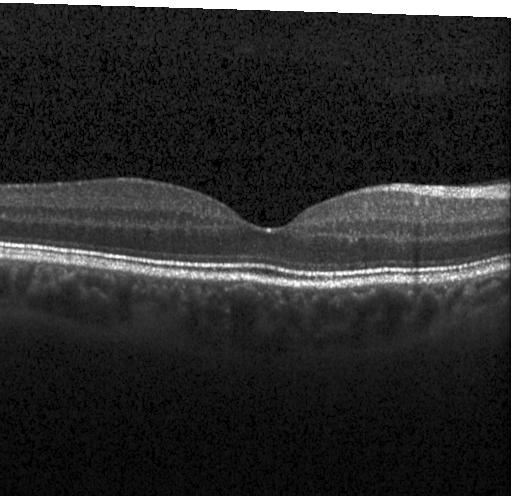
Finding: no choroidal neovascularization, diabetic macular edema, or drusen.